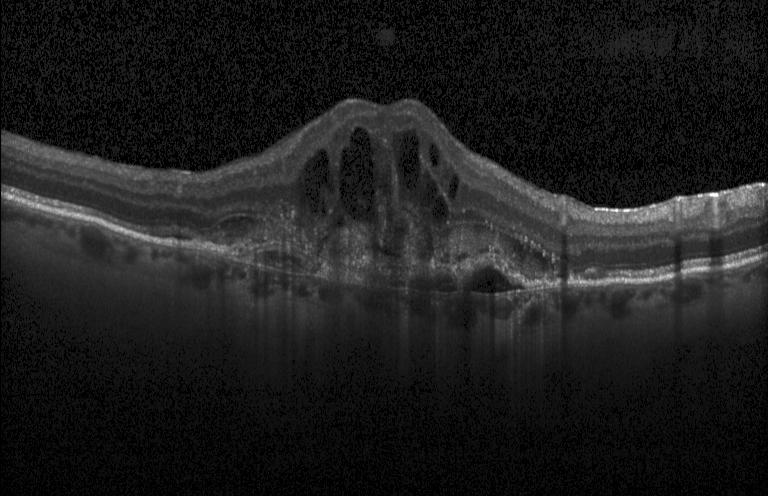

Spectral-domain OCT; optical coherence tomography scan; acquired on a Heidelberg Spectralis; horizontal scan through the fovea. This B-scan demonstrates a choroidal neovascular membrane.